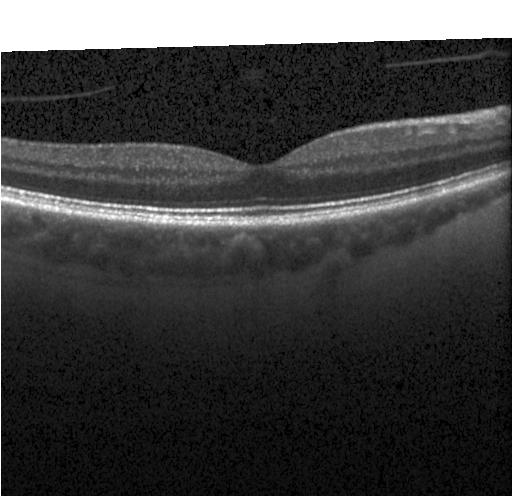
Impression: no CNV, no DME, and no drusen.